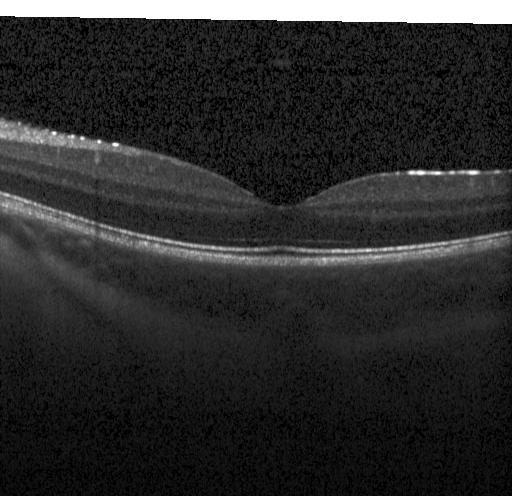 Optical coherence tomography B-scan; Heidelberg Spectralis; through the macula — Diagnosis: no CNV, no DME, and no drusen.